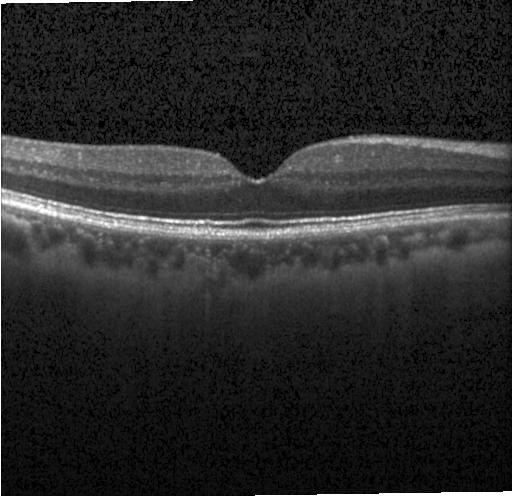
Optical coherence tomography scan — Impression: no choroidal neovascularization, no diabetic macular edema, and no drusen.